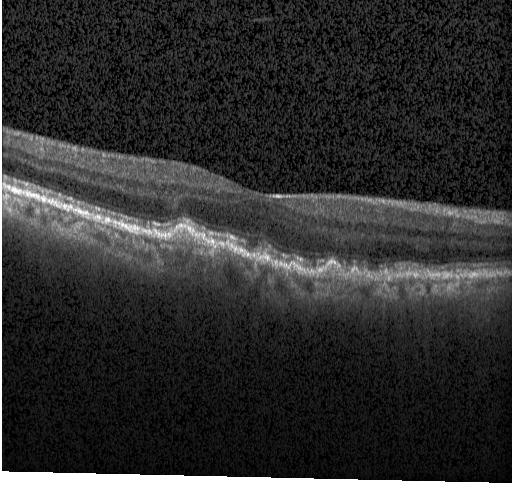
Heidelberg Spectralis, OCT line scan, SD-OCT, through the macula
OCT finding: multiple drusen.